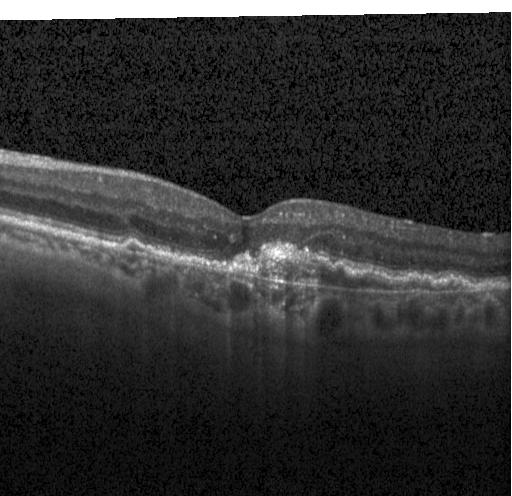

OCT finding: a choroidal neovascular membrane.